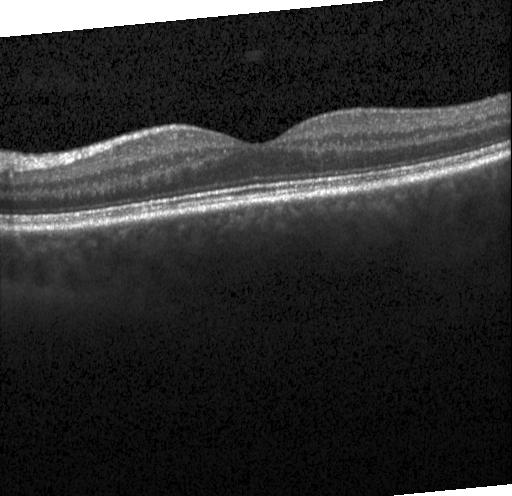 Assessment: no CNV, DME, or drusen.